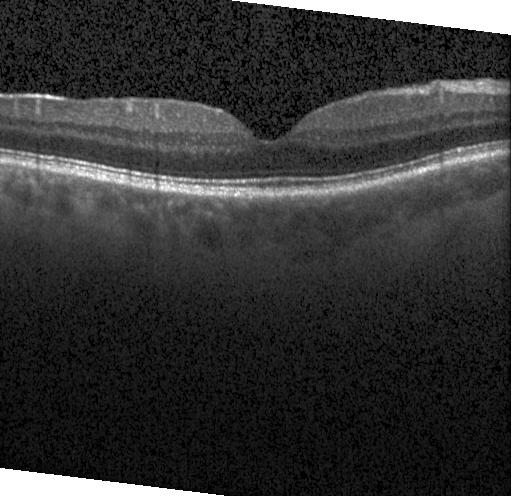

Retinal OCT cross-section. Impression: neither CNV, DME, nor drusen.